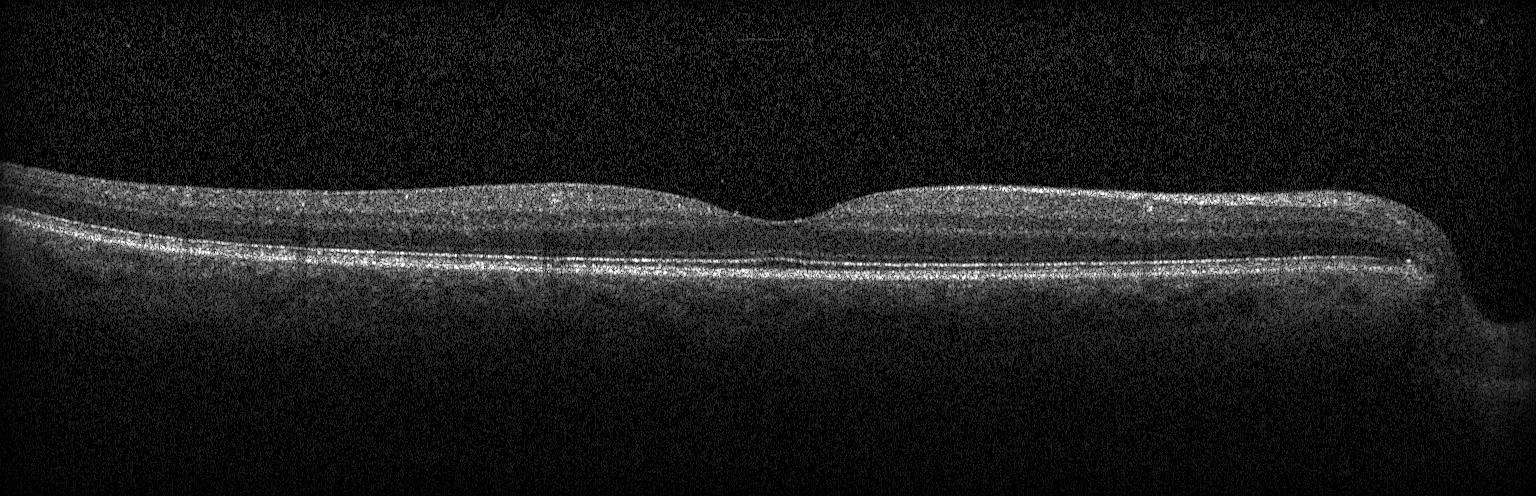 Optical coherence tomography scan
Diagnosis: neither choroidal neovascularization, diabetic macular edema, nor drusen.